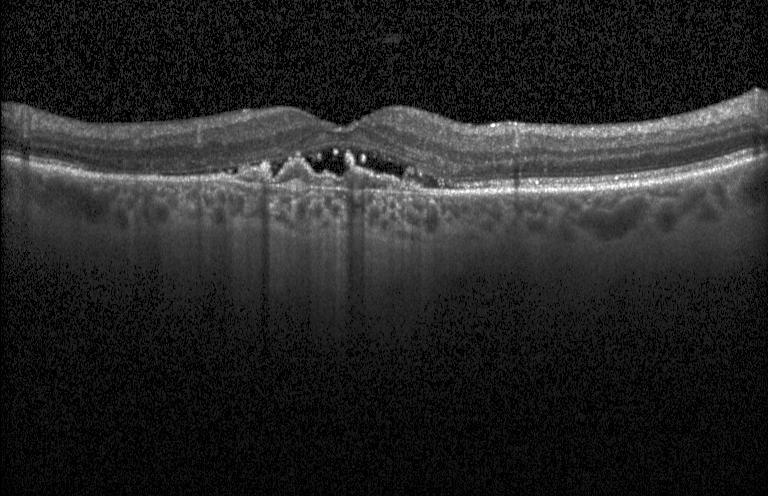 Heidelberg Spectralis OCT system · retinal OCT B-scan
Finding: choroidal neovascularization (CNV).